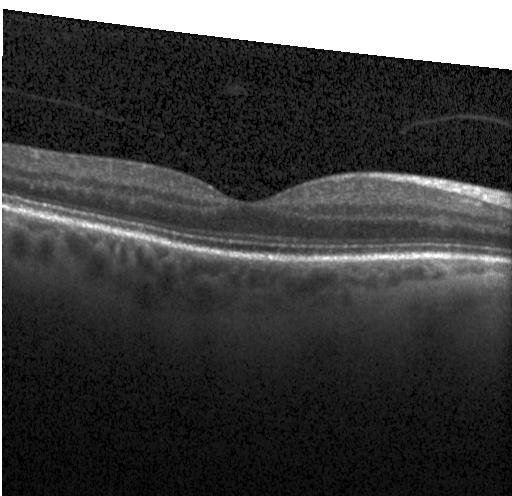 Optical coherence tomography scan, macular scan, SD-OCT.
Diagnosis: no choroidal neovascularization, no diabetic macular edema, and no drusen.